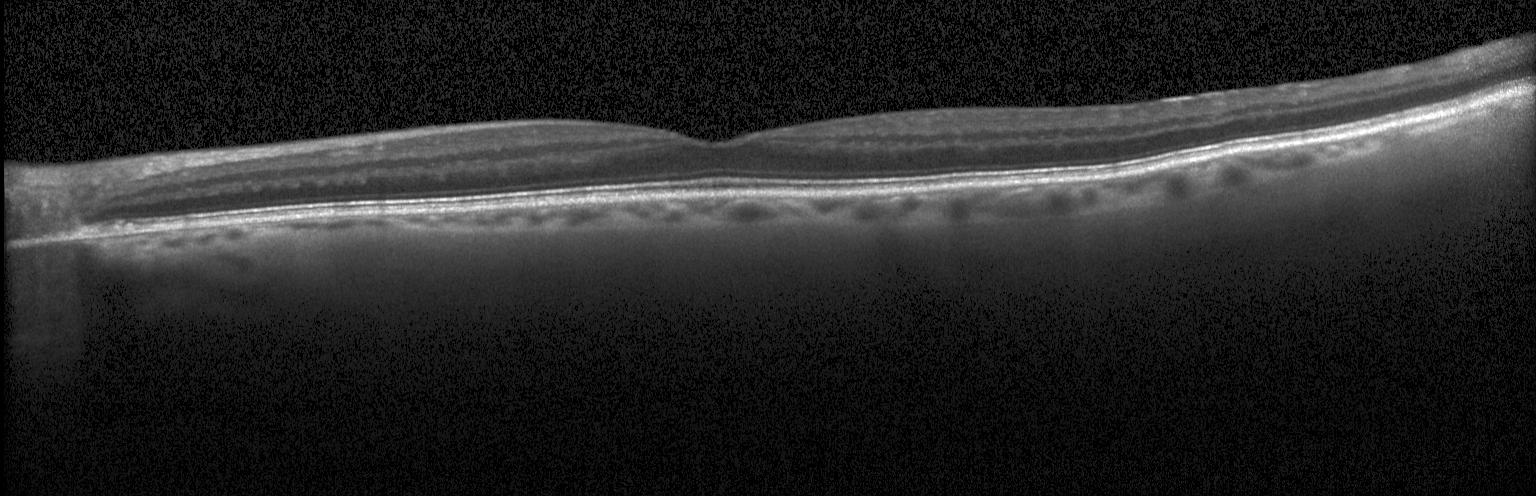

OCT B-scan, SD-OCT, Heidelberg Spectralis OCT system. Impression: no choroidal neovascularization, diabetic macular edema, or drusen.